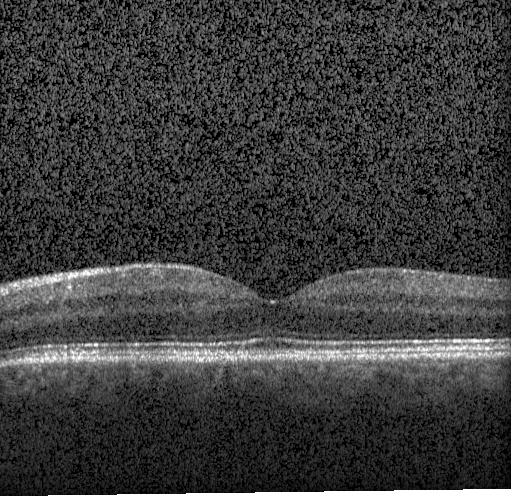
Fovea-centered, spectral-domain OCT, Heidelberg Spectralis, OCT line scan.
Assessment: no choroidal neovascularization, no diabetic macular edema, and no drusen.